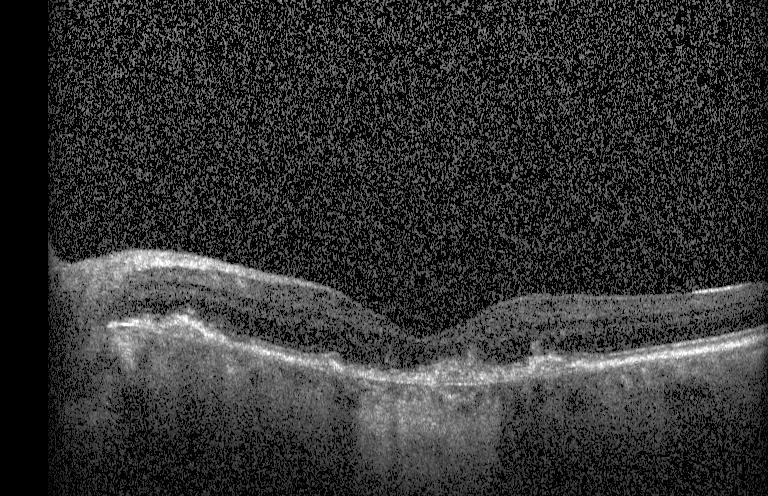

Diagnosis: a choroidal neovascular membrane.